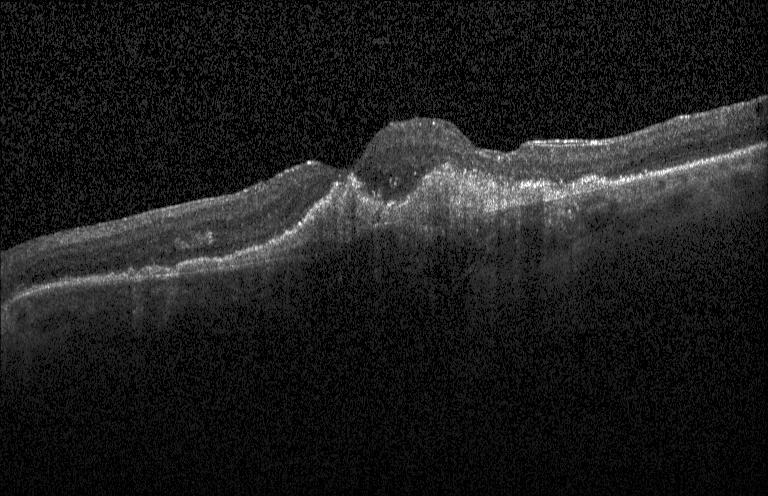

Horizontal scan through the fovea, retinal OCT B-scan.
This B-scan demonstrates a choroidal neovascular membrane.